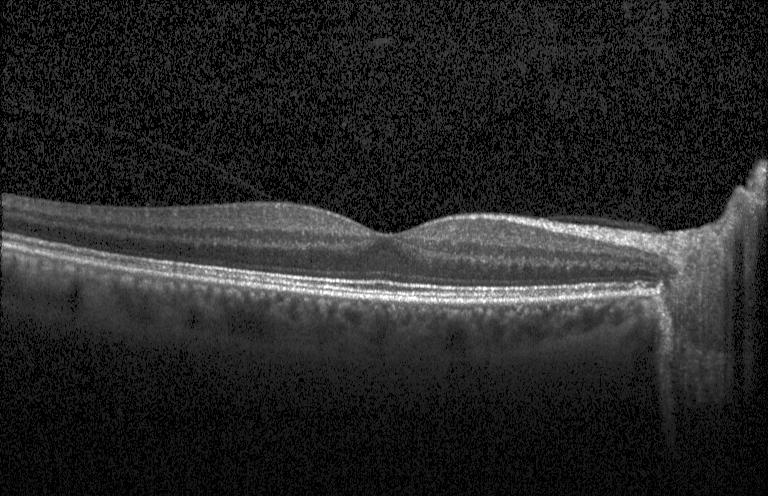

Neither choroidal neovascularization, diabetic macular edema, nor drusen.